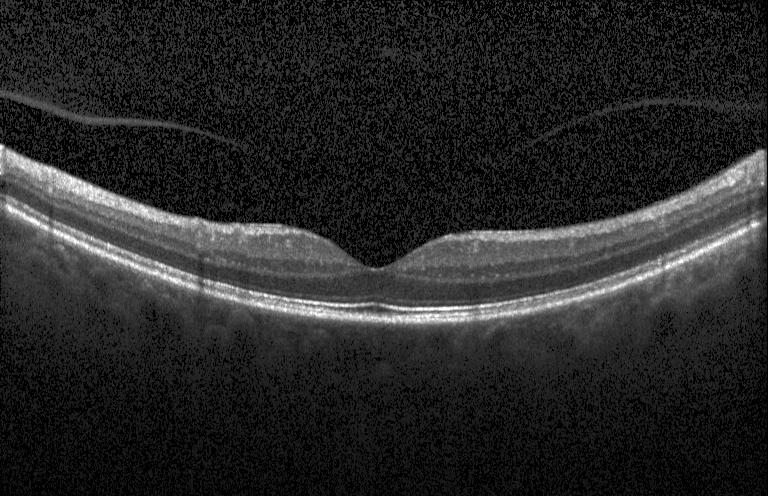 Fovea-centered; retinal OCT cross-section.
Diagnosis: neither CNV, DME, nor drusen.